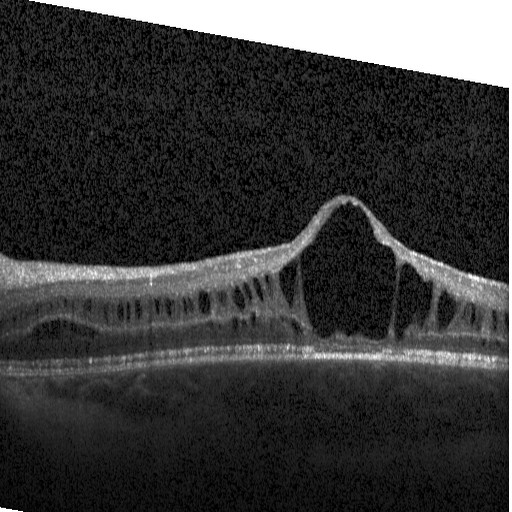
Impression: DME.